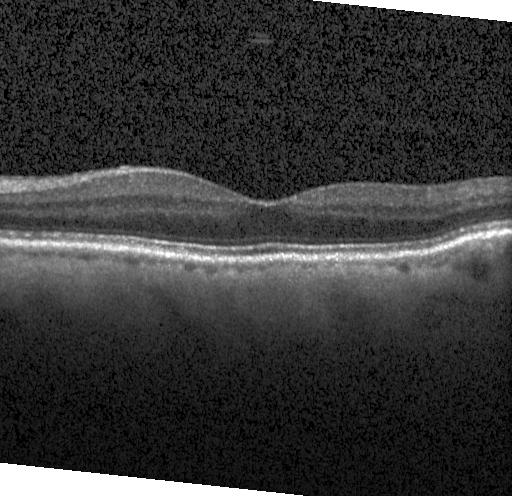

Instrument: Heidelberg Spectralis · retinal OCT B-scan
Impression: no choroidal neovascularization, diabetic macular edema, or drusen.